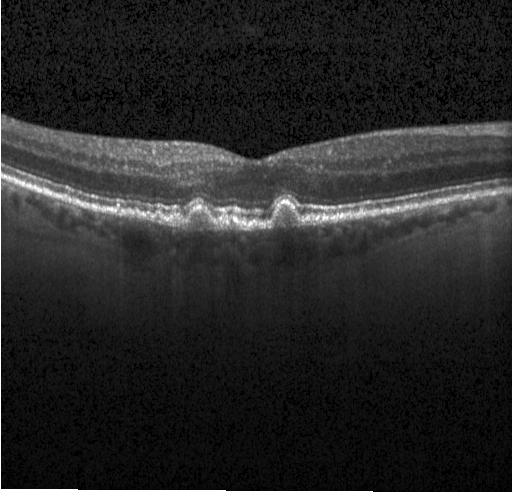

Finding: multiple drusen.